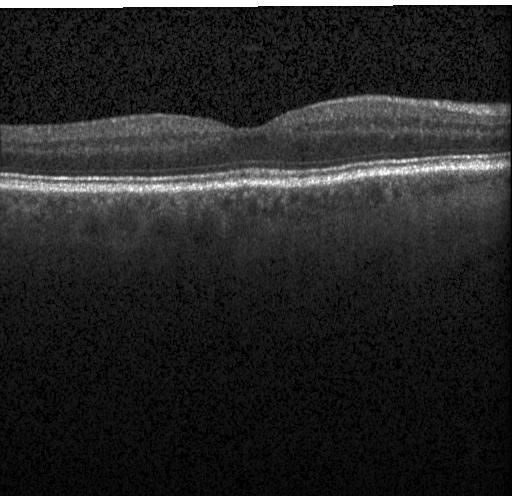
OCT line scan · spectral-domain OCT · centered on the fovea. This B-scan demonstrates no evidence of choroidal neovascularization, diabetic macular edema, or drusen.